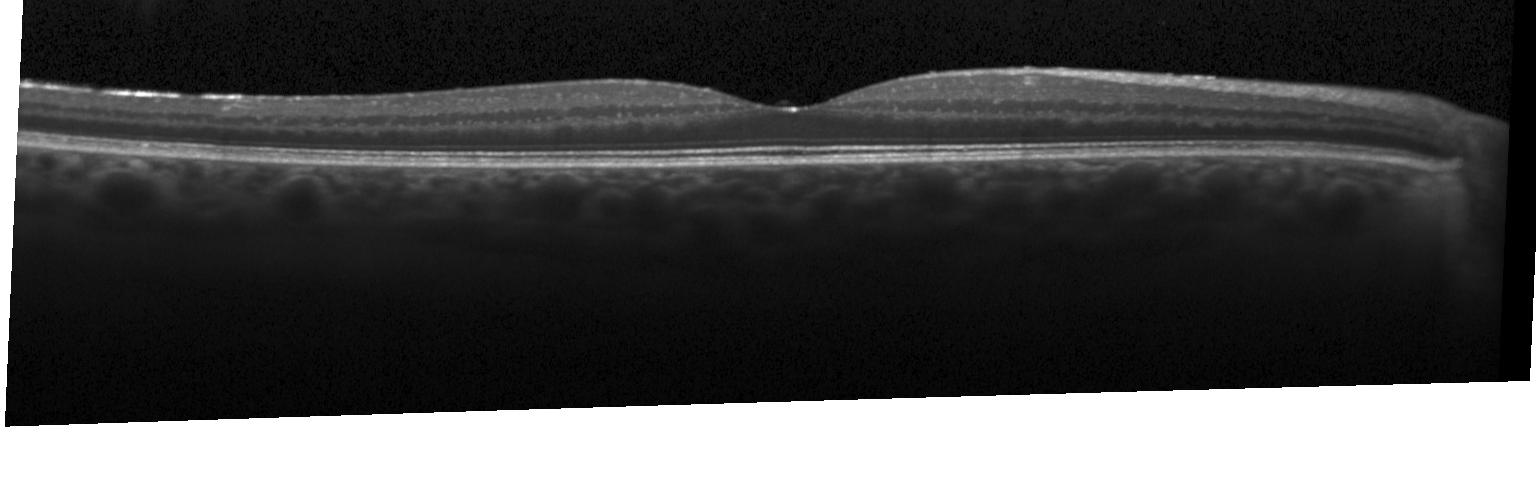 Optical coherence tomography scan, Heidelberg Spectralis, horizontal scan through the fovea
Assessment: no evidence of CNV, DME, or drusen.